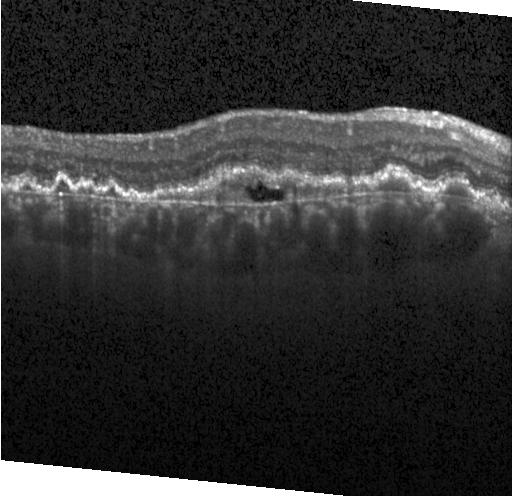 Macular scan; OCT line scan.
Macular OCT: a choroidal neovascular membrane.